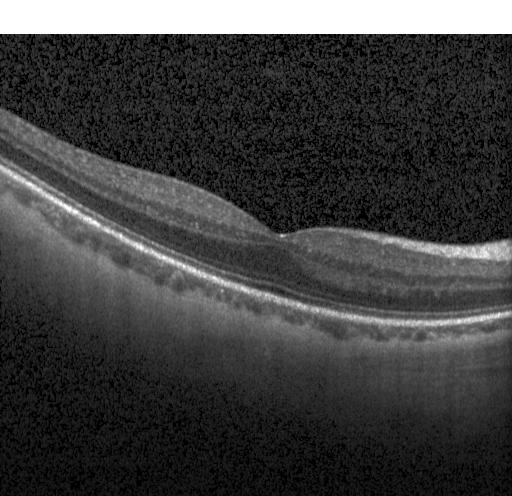 Acquired on a Heidelberg Spectralis · centered on the fovea · spectral-domain optical coherence tomography · OCT line scan. Macular OCT: no choroidal neovascularization, diabetic macular edema, or drusen.